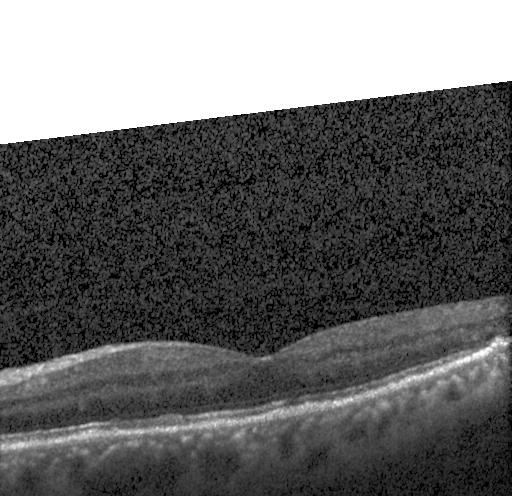

Finding: sub-RPE drusenoid deposits.